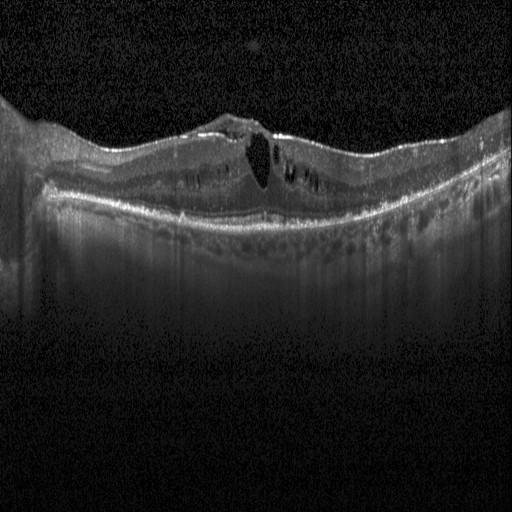 OCT B-scan.
Diagnosis: diabetic macular edema.